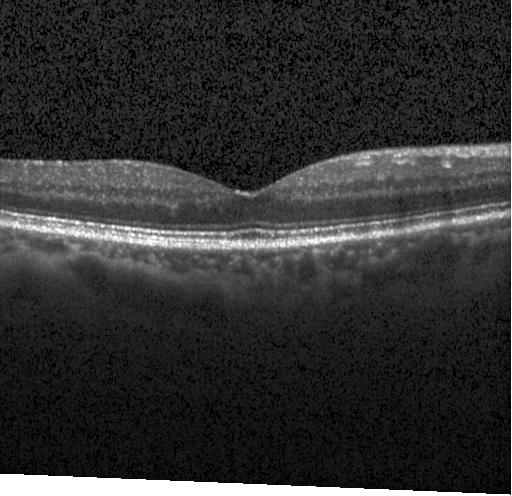
Through the macula. Heidelberg Spectralis OCT system. OCT line scan.
Finding: no evidence of choroidal neovascularization, diabetic macular edema, or drusen.